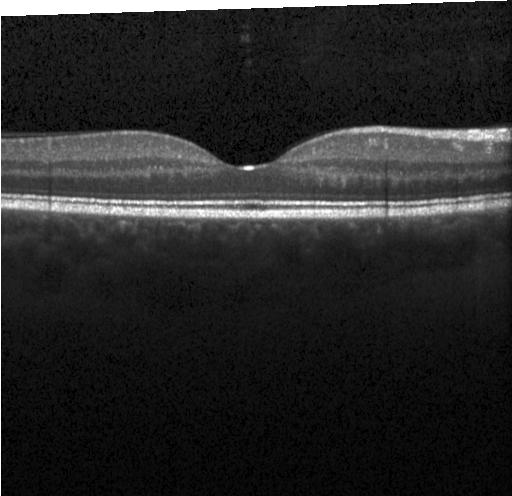
Fovea-centered. Optical coherence tomography scan. Spectral-domain optical coherence tomography. Heidelberg Spectralis — Macular OCT: no evidence of choroidal neovascularization, diabetic macular edema, or drusen.